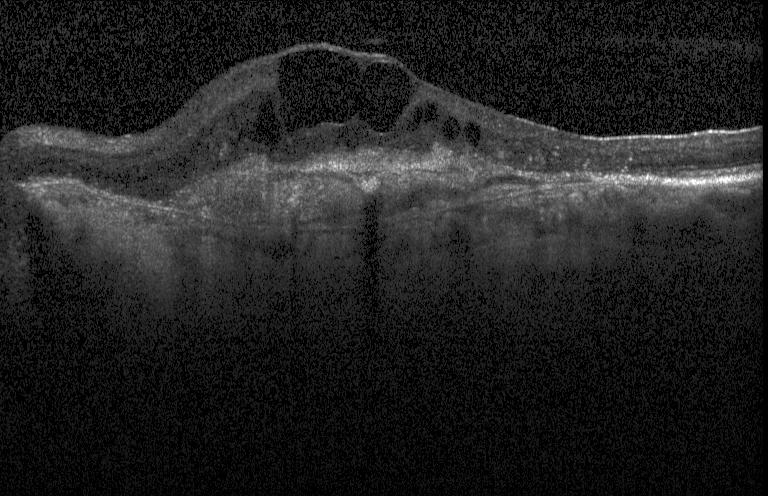

OCT line scan, acquired on a Heidelberg Spectralis, spectral-domain OCT, through the macula — Finding: a choroidal neovascular membrane.